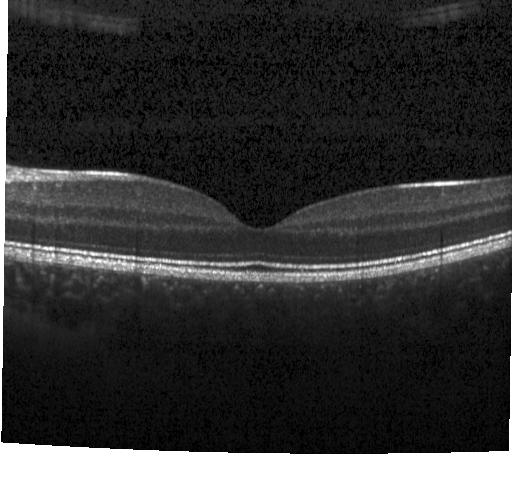

Spectral-domain OCT B-scan: no CNV, DME, or drusen.